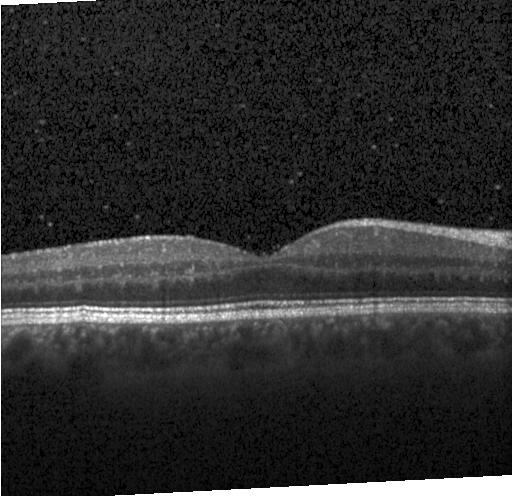 OCT line scan. SD-OCT. Fovea-centered. Heidelberg Spectralis OCT system
This B-scan demonstrates neither choroidal neovascularization, diabetic macular edema, nor drusen.